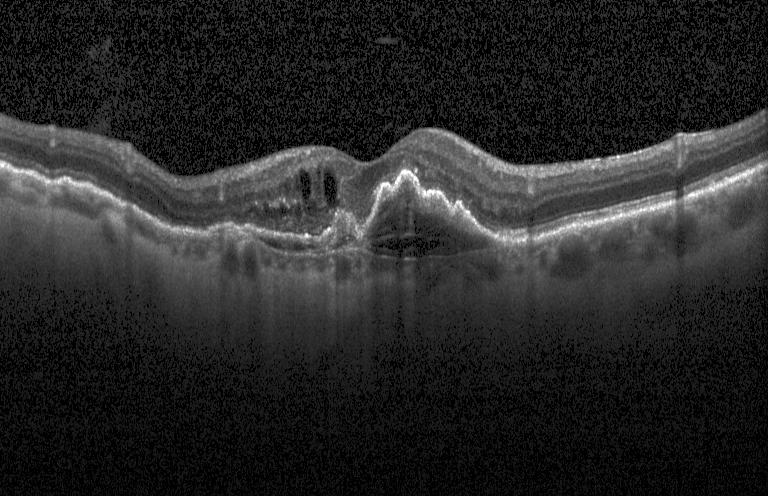

Spectral-domain optical coherence tomography, optical coherence tomography scan, centered on the fovea — Impression: choroidal neovascularization.